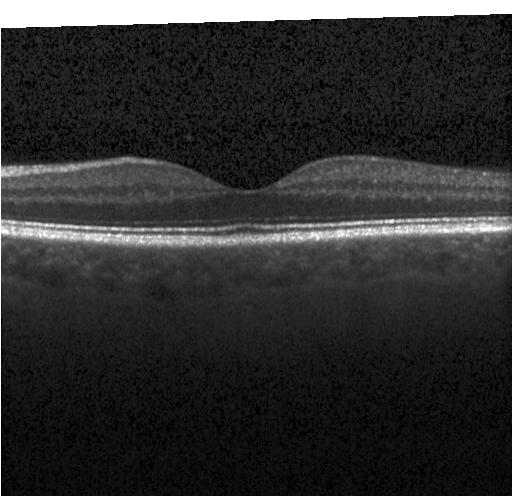

Retinal OCT cross-section showing no CNV, DME, or drusen.